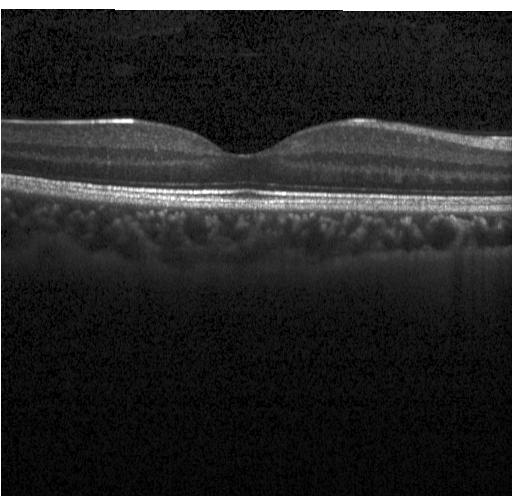

Optical coherence tomography scan — Diagnosis: no evidence of choroidal neovascularization, diabetic macular edema, or drusen.